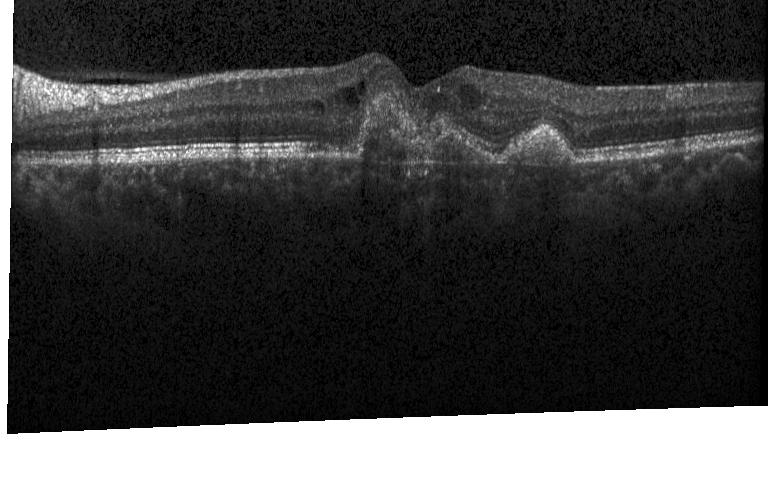

Acquired on a Heidelberg Spectralis · OCT line scan · through the macula · spectral-domain OCT — Impression: CNV.